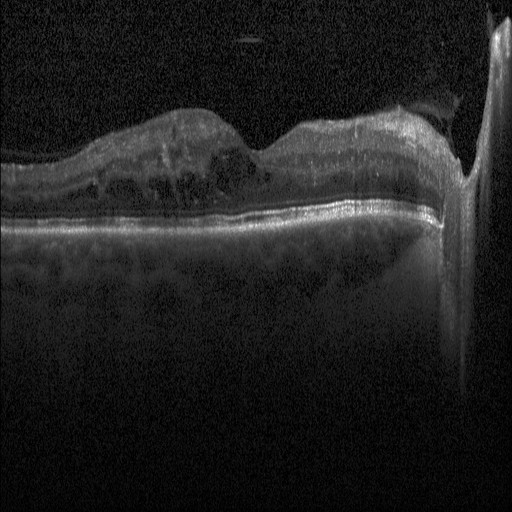

Macular OCT: DME.